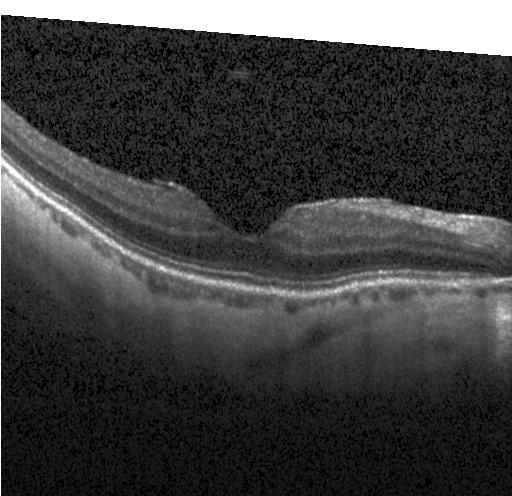
Retinal OCT B-scan
The scan shows no choroidal neovascularization, diabetic macular edema, or drusen.